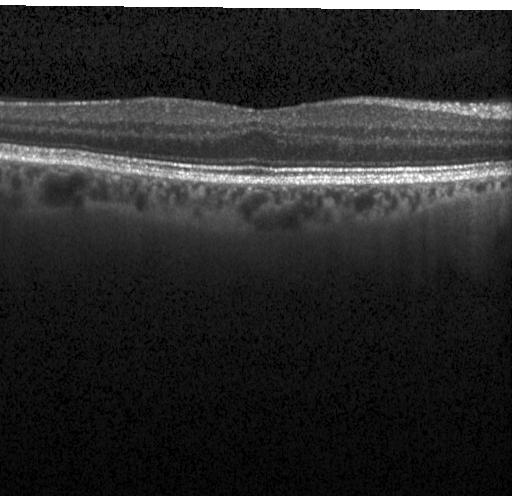
Impression: no CNV, no DME, and no drusen.